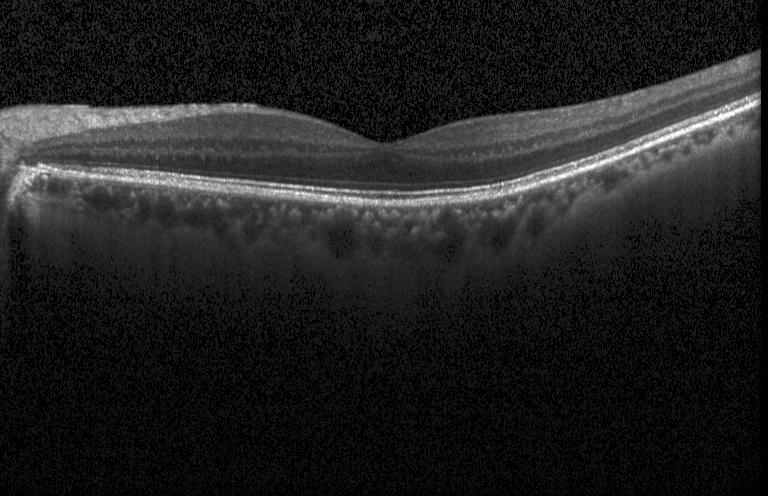
OCT B-scan. SD-OCT
This B-scan demonstrates no evidence of choroidal neovascularization, diabetic macular edema, or drusen.